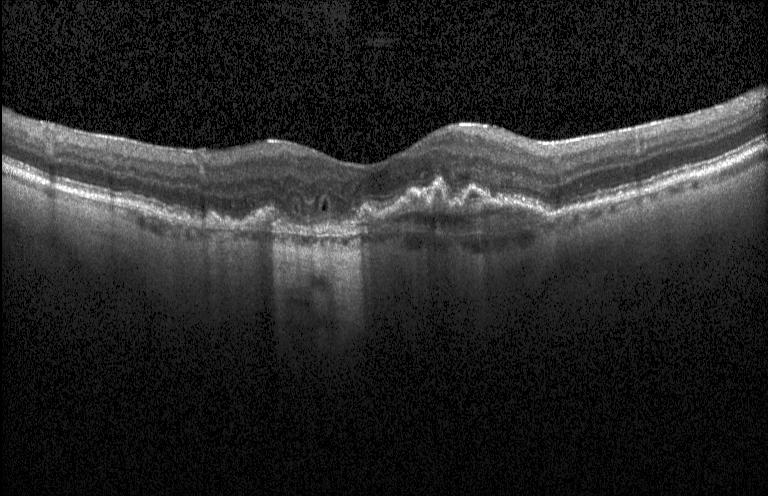
Instrument: Heidelberg Spectralis · OCT line scan · SD-OCT
Macular OCT: a choroidal neovascular membrane.